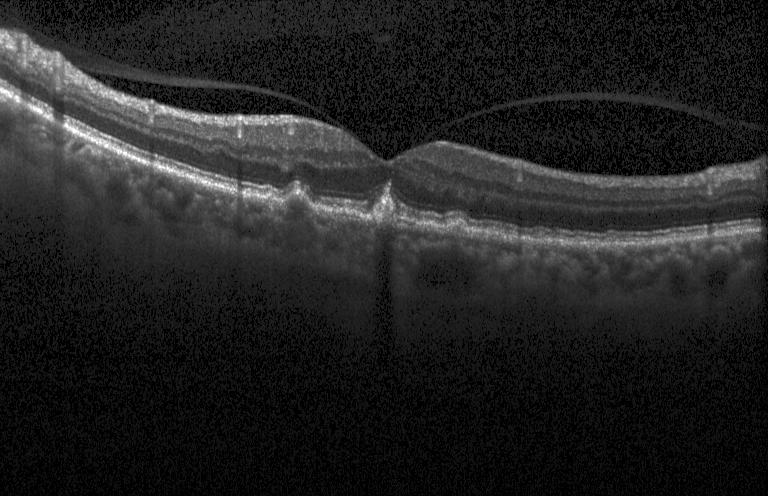 OCT B-scan.
Finding: drusen.